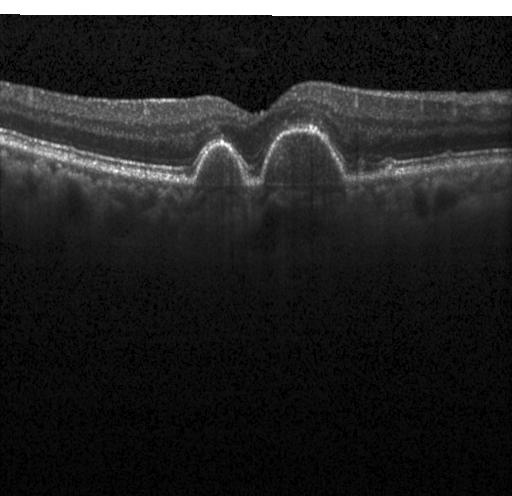 Dx: sub-RPE drusenoid deposits.